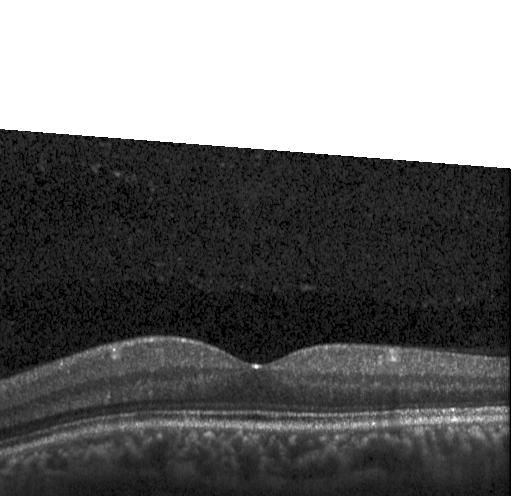
Impression: no choroidal neovascularization, diabetic macular edema, or drusen.